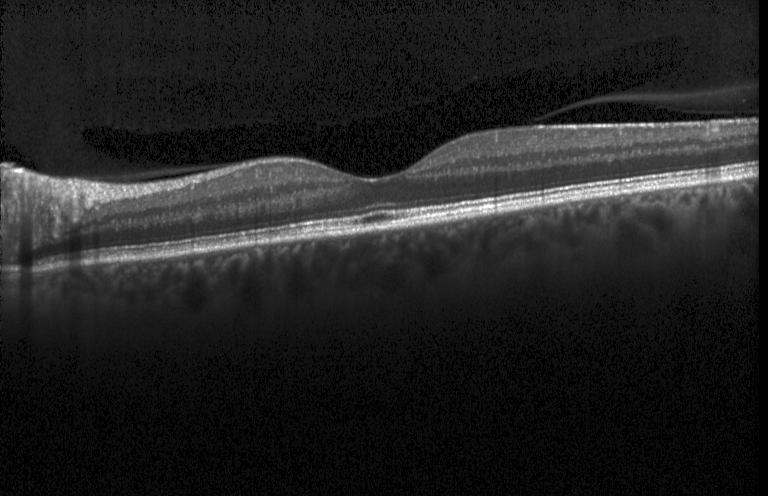

Instrument: Heidelberg Spectralis. Retinal OCT cross-section. Spectral-domain optical coherence tomography. Fovea-centered — Assessment: no evidence of choroidal neovascularization, diabetic macular edema, or drusen.